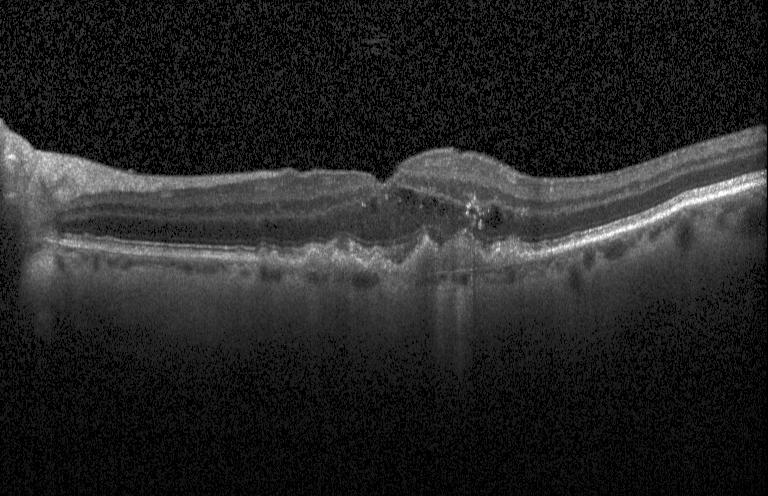

The scan shows a choroidal neovascular membrane.